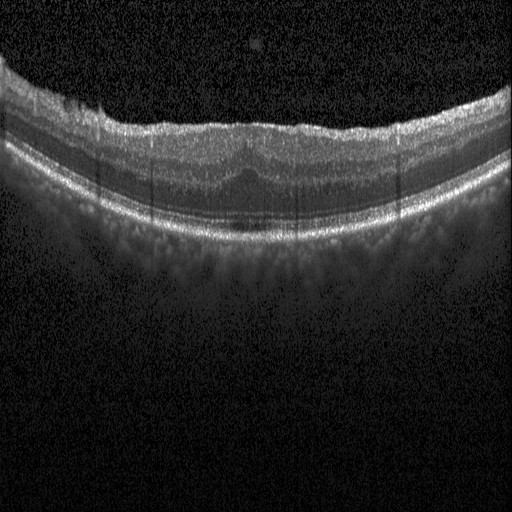
OCT line scan. Finding: diabetic macular edema (DME).